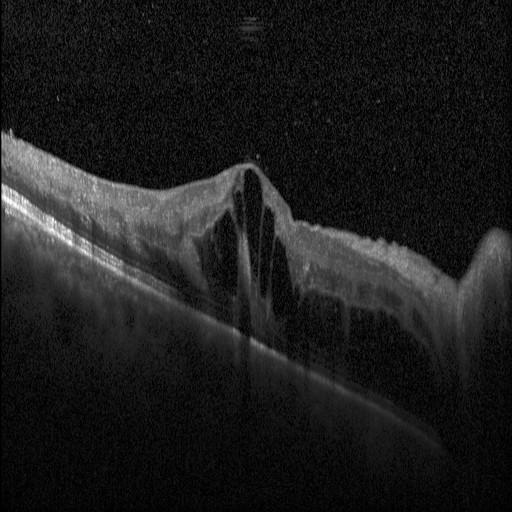 Retinal OCT cross-section showing diabetic macular edema.